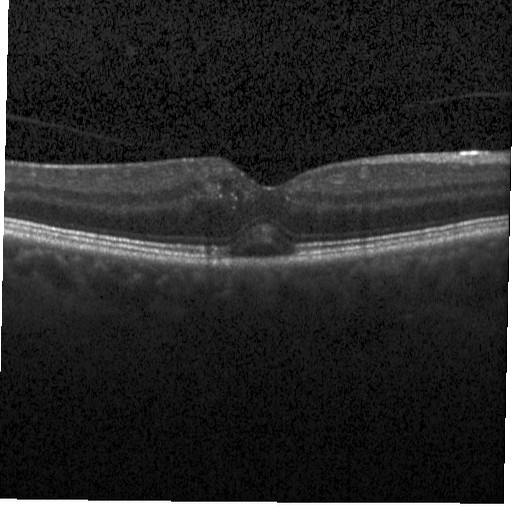
Finding: diabetic macular edema.